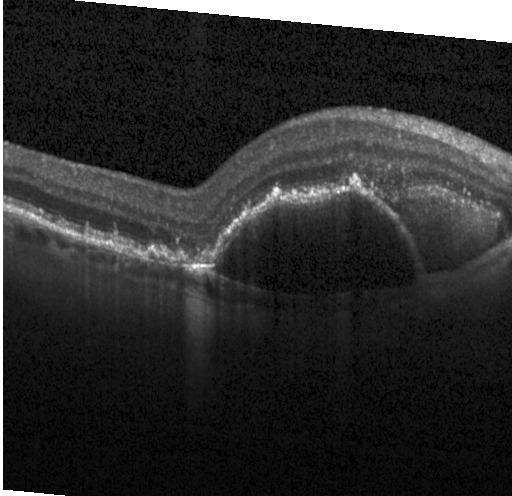
Fovea-centered. OCT B-scan
Dx: choroidal neovascularization (CNV).